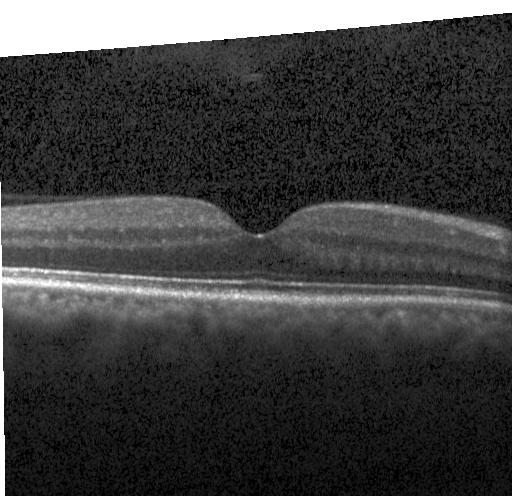
Retinal OCT cross-section showing neither CNV, DME, nor drusen.